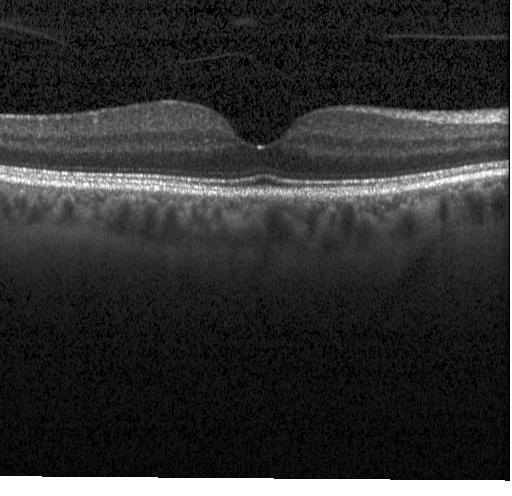
Optical coherence tomography B-scan. Macular scan. Heidelberg Spectralis OCT system. Spectral-domain OCT. OCT finding: no choroidal neovascularization, no diabetic macular edema, and no drusen.